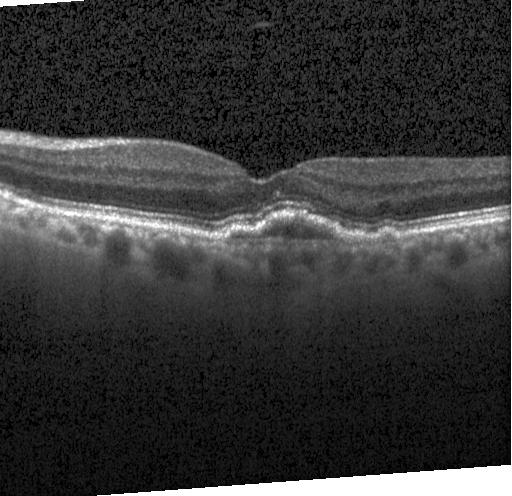
Spectral-domain optical coherence tomography. Fovea-centered. Heidelberg Spectralis OCT system. OCT line scan — Impression: choroidal neovascularization (CNV).